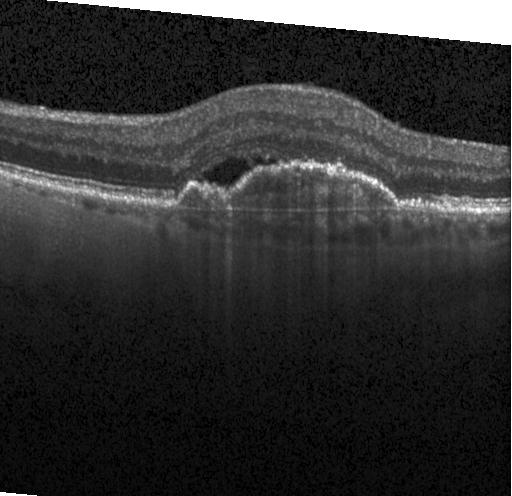

Optical coherence tomography scan · instrument: Heidelberg Spectralis · spectral-domain optical coherence tomography · horizontal scan through the fovea.
This B-scan demonstrates a choroidal neovascular membrane.